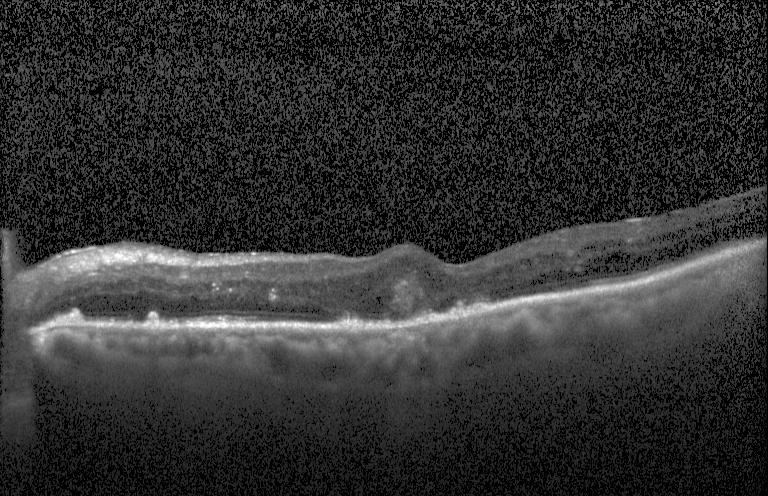

OCT B-scan · macular scan · spectral-domain OCT
This B-scan demonstrates a choroidal neovascular membrane.